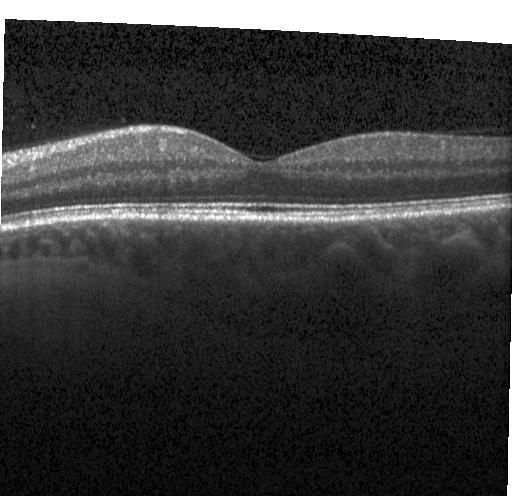

SD-OCT; OCT line scan — Macular OCT: no choroidal neovascularization, no diabetic macular edema, and no drusen.